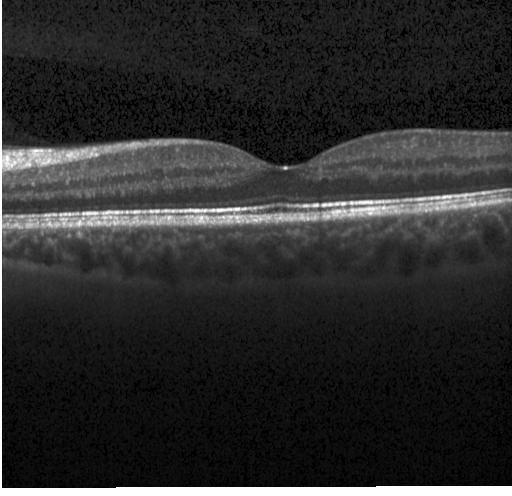
OCT B-scan · spectral-domain optical coherence tomography.
This B-scan demonstrates no CNV, no DME, and no drusen.